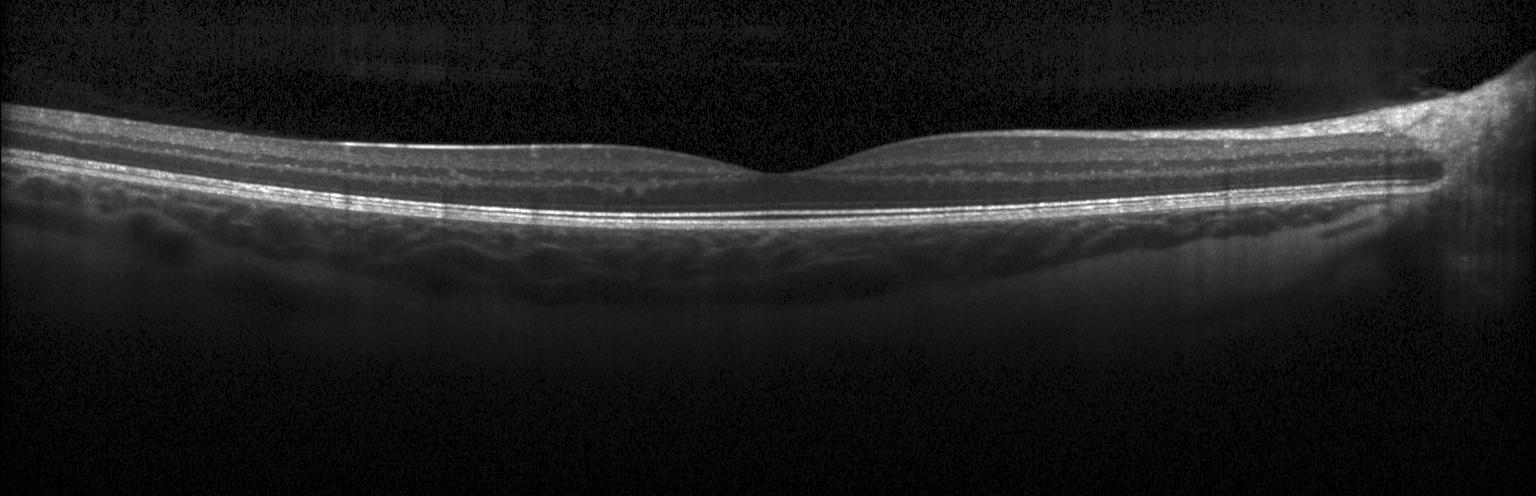

Retinal OCT cross-section. Impression: no CNV, DME, or drusen.